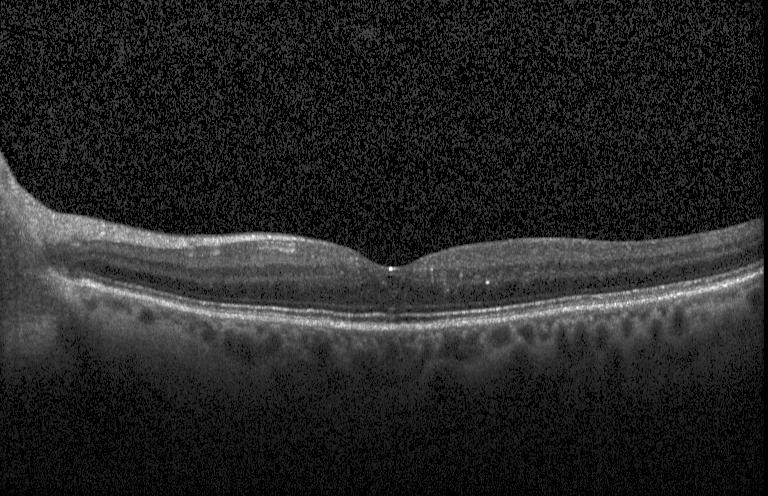 Centered on the fovea · spectral-domain optical coherence tomography · optical coherence tomography scan.
Macular OCT: no CNV, no DME, and no drusen.